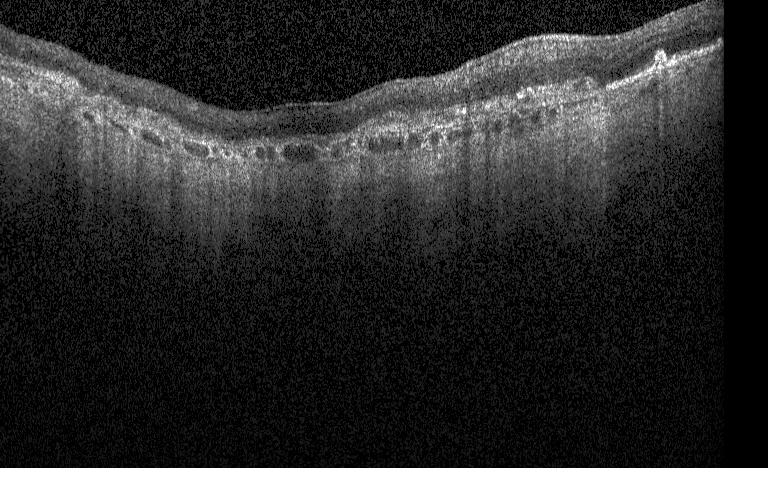

Centered on the fovea; Heidelberg Spectralis OCT system; OCT line scan; spectral-domain optical coherence tomography. The scan shows a choroidal neovascular membrane.